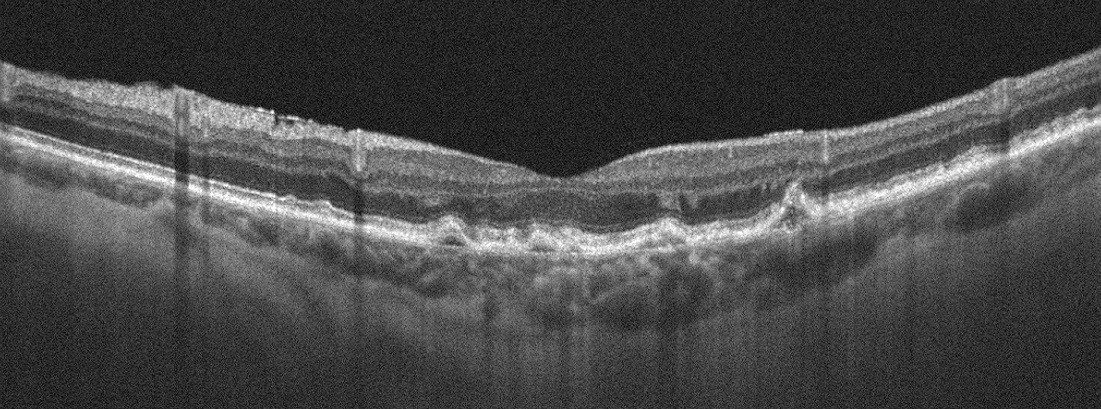

Macular OCT: age-related macular degeneration (AMD).